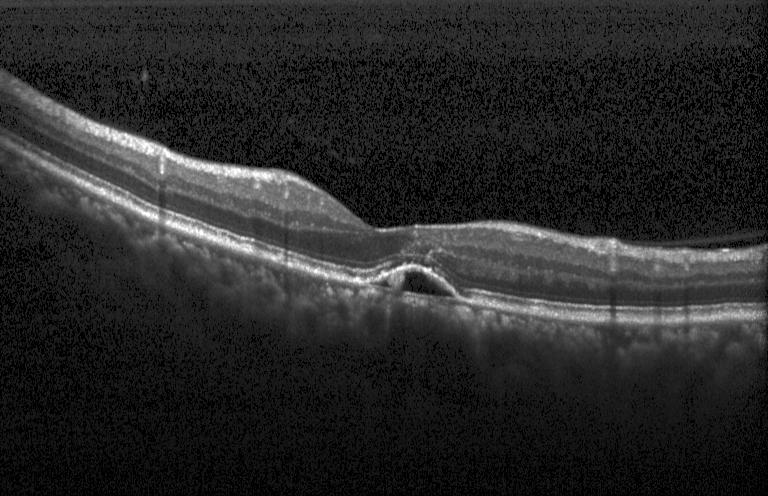 Spectral-domain optical coherence tomography · OCT line scan
Impression: a choroidal neovascular membrane.